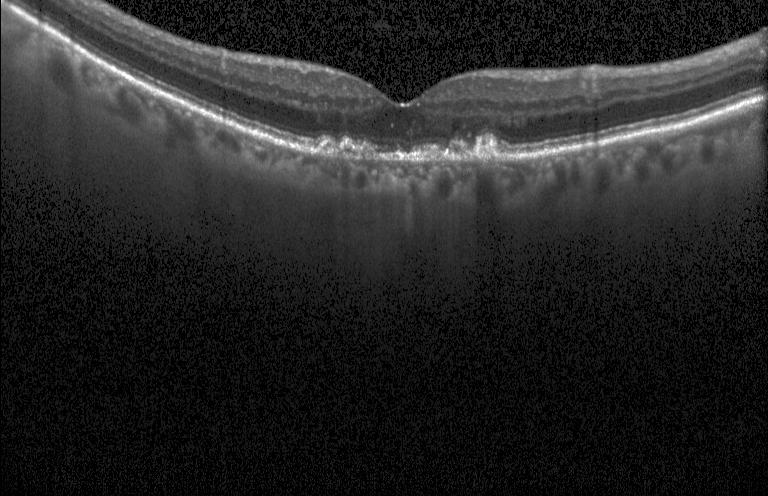
Spectral-domain optical coherence tomography · macular scan · retinal OCT cross-section · instrument: Heidelberg Spectralis — Diagnosis: multiple drusen.